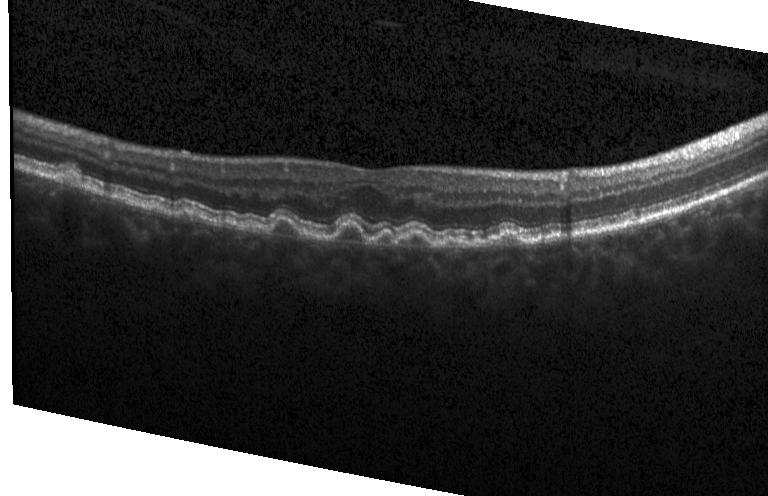 OCT line scan — This B-scan demonstrates sub-RPE drusenoid deposits.